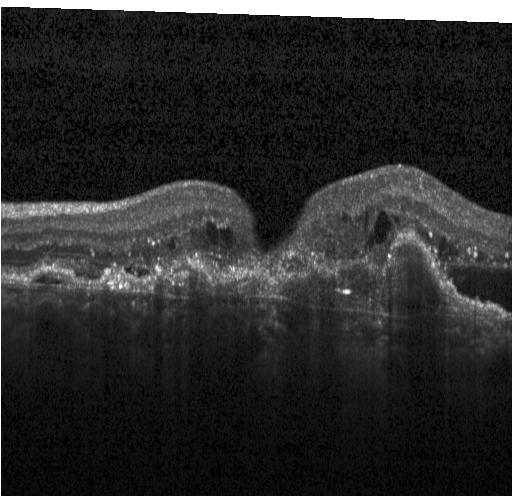
Impression: a choroidal neovascular membrane.